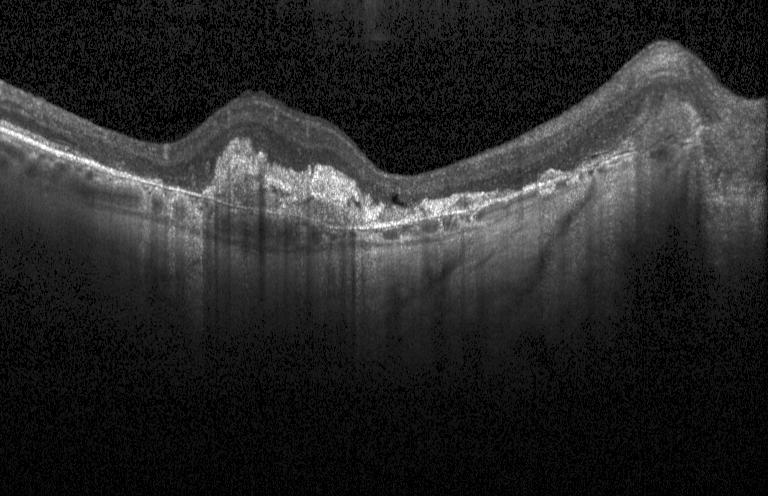 Impression: choroidal neovascularization (CNV).